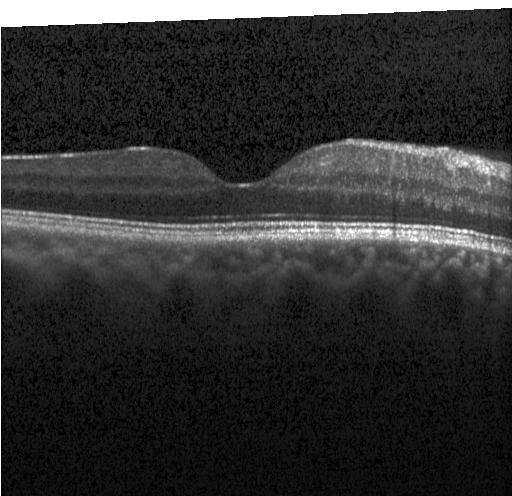
Retinal OCT cross-section. Heidelberg Spectralis.
Finding: no evidence of choroidal neovascularization, diabetic macular edema, or drusen.